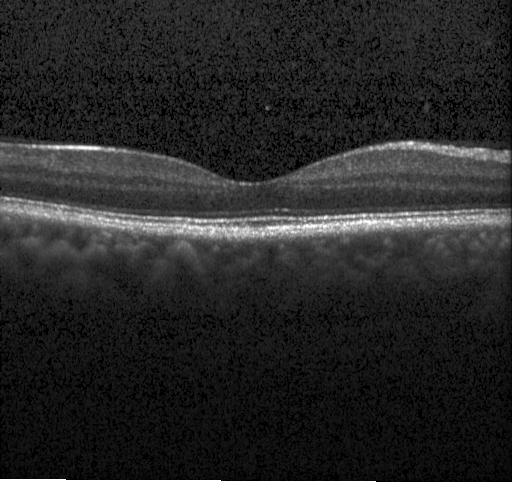 Retinal OCT B-scan.
The scan shows no choroidal neovascularization, diabetic macular edema, or drusen.